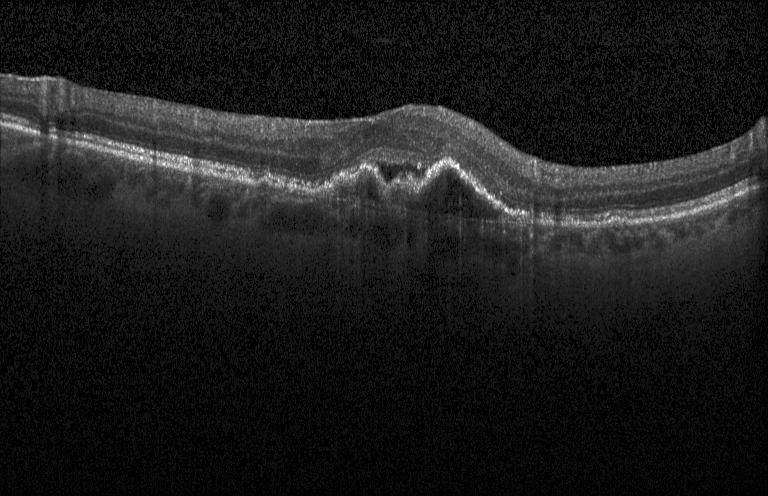 OCT finding: CNV.